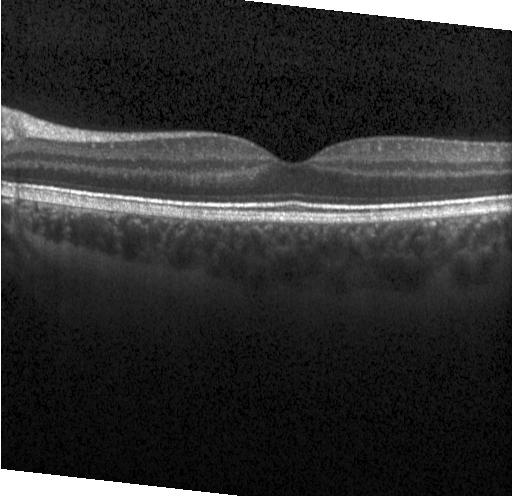

OCT line scan, SD-OCT, acquired on a Heidelberg Spectralis, centered on the fovea.
Macular OCT: no CNV, no DME, and no drusen.